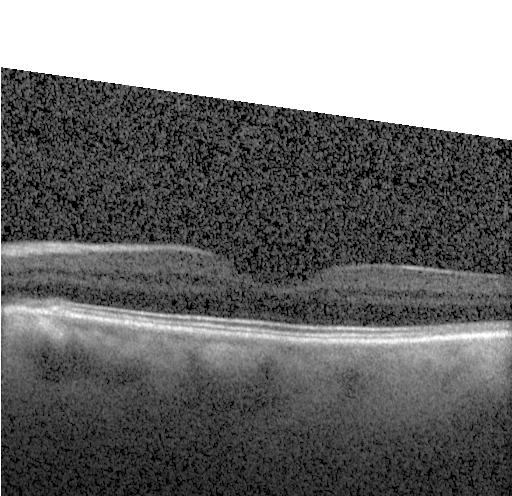
Fovea-centered; SD-OCT; Heidelberg Spectralis; OCT line scan.
Assessment: neither choroidal neovascularization, diabetic macular edema, nor drusen.